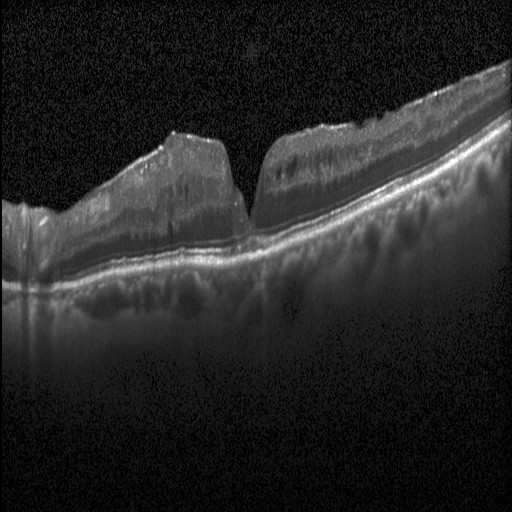

Through the macula. Heidelberg Spectralis. Optical coherence tomography B-scan. Impression: DME.